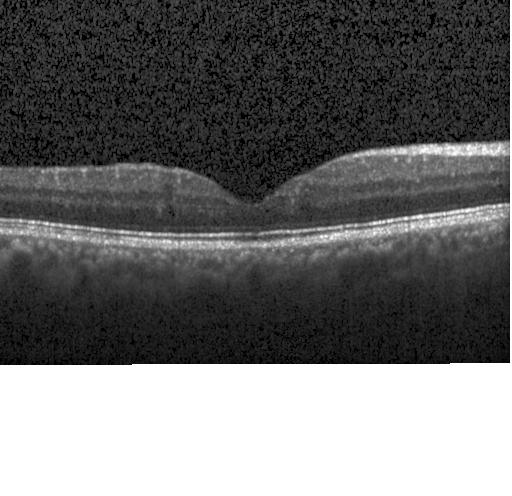

Optical coherence tomography scan. Diagnosis: no evidence of choroidal neovascularization, diabetic macular edema, or drusen.